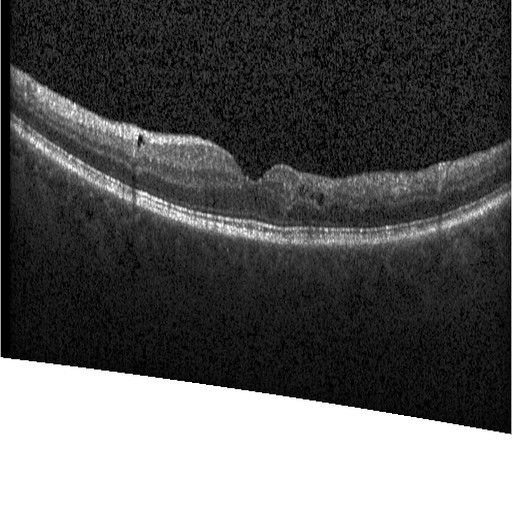 Instrument: Heidelberg Spectralis · spectral-domain OCT · retinal OCT B-scan · macular scan — Macular OCT: DME.